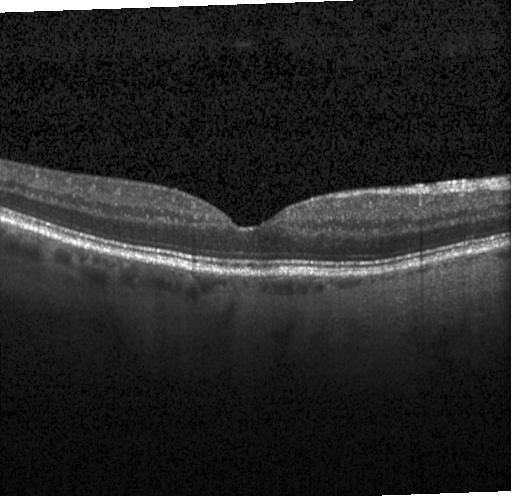 Macular OCT demonstrating no choroidal neovascularization, diabetic macular edema, or drusen.